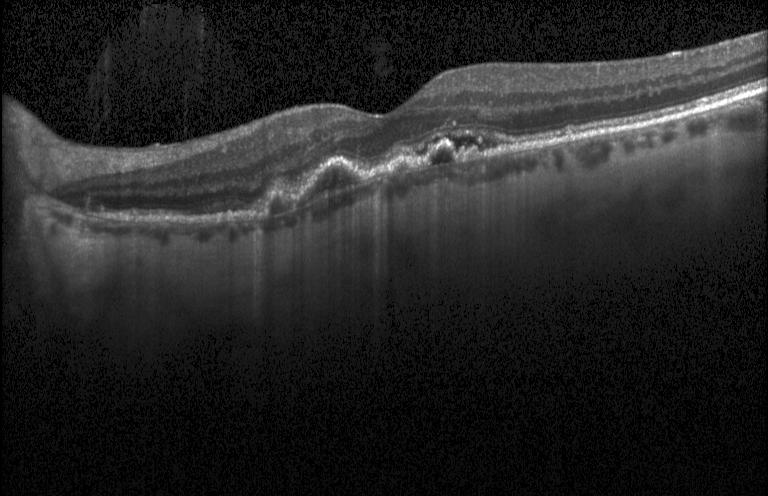 Spectral-domain OCT B-scan: a choroidal neovascular membrane.